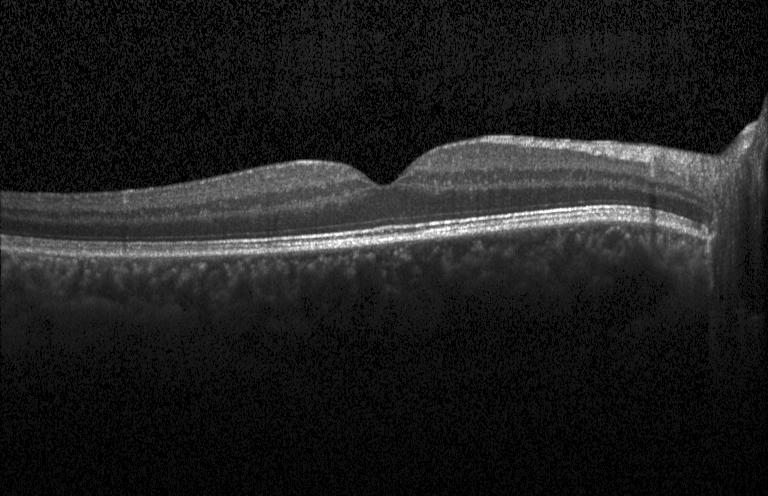
OCT line scan
OCT finding: no choroidal neovascularization, no diabetic macular edema, and no drusen.